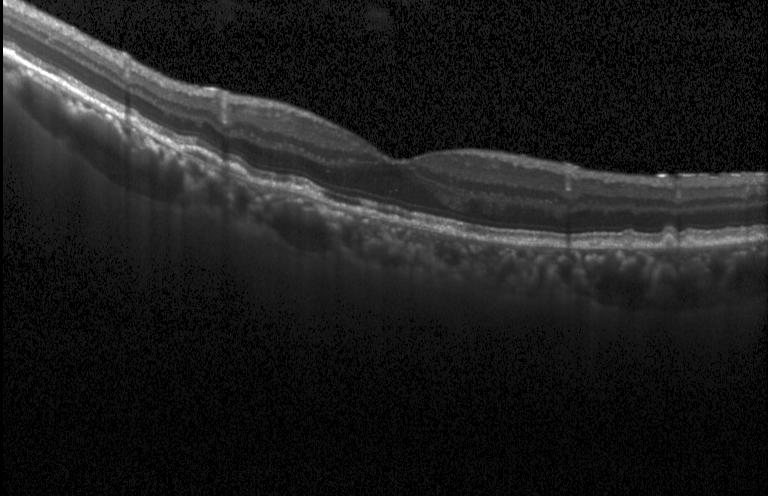 Centered on the fovea, SD-OCT, OCT line scan.
Finding: sub-RPE drusenoid deposits.